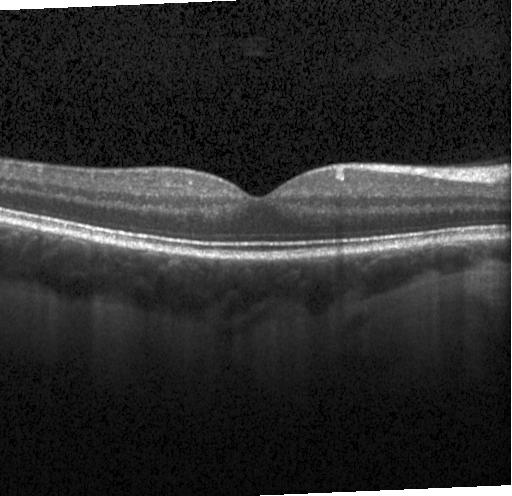
The scan shows no evidence of CNV, DME, or drusen.